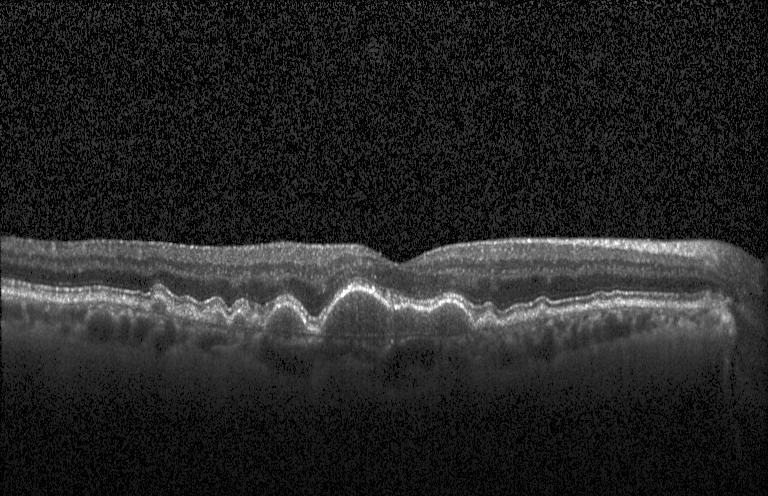
Finding: sub-RPE drusenoid deposits.